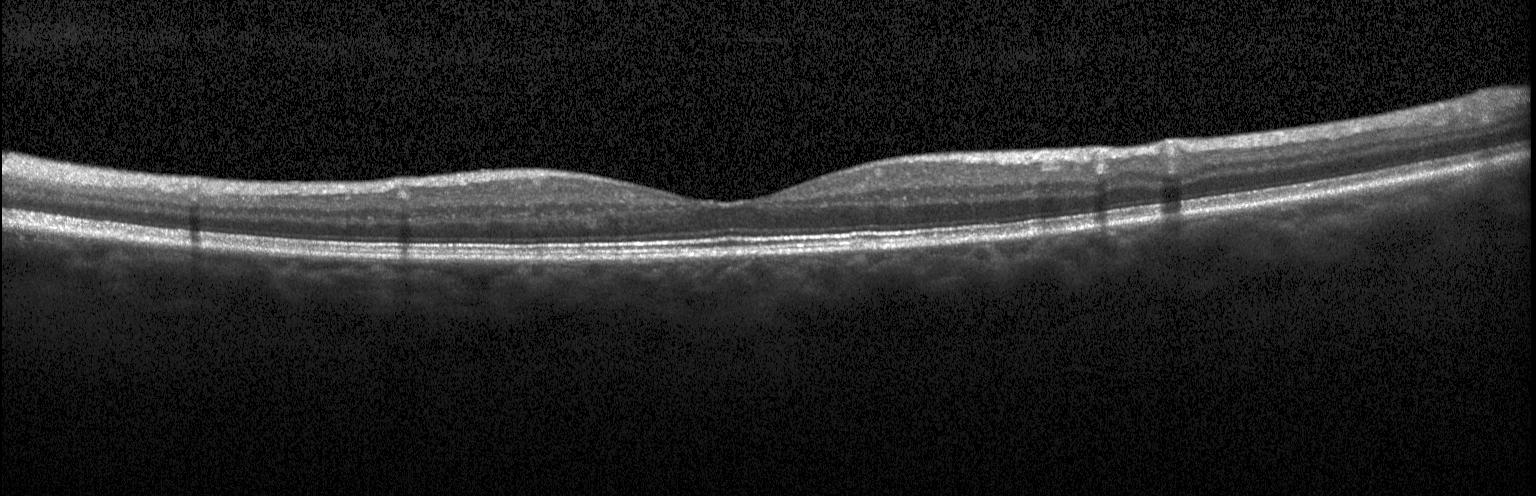

SD-OCT; retinal OCT B-scan
Dx: no CNV, DME, or drusen.